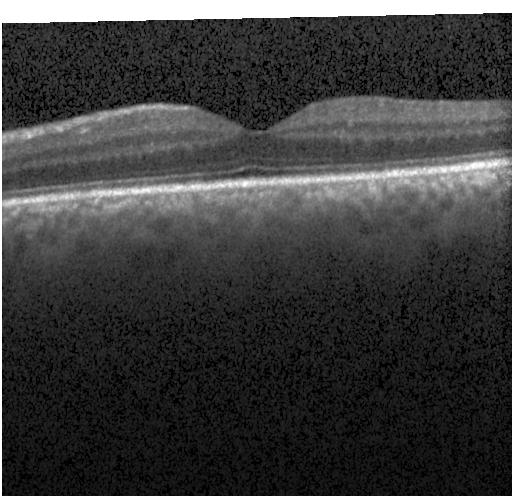

Acquired on a Heidelberg Spectralis, SD-OCT, optical coherence tomography B-scan.
Finding: no evidence of CNV, DME, or drusen.